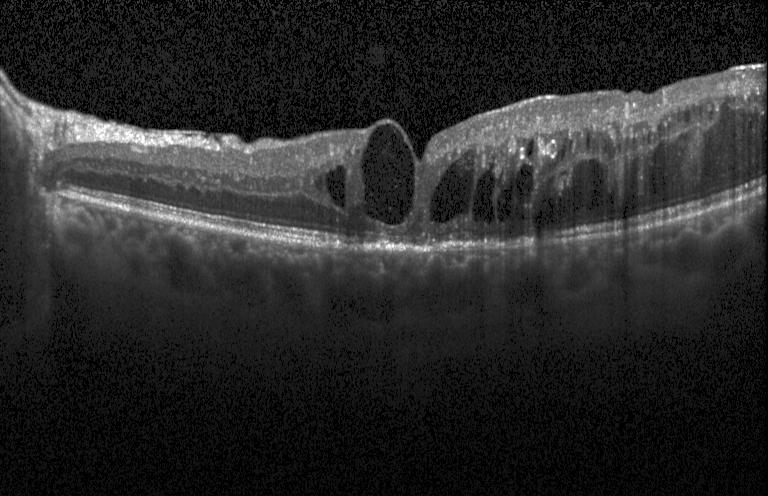

Spectral-domain optical coherence tomography, through the macula, OCT B-scan, Heidelberg Spectralis OCT system
Impression: DME.